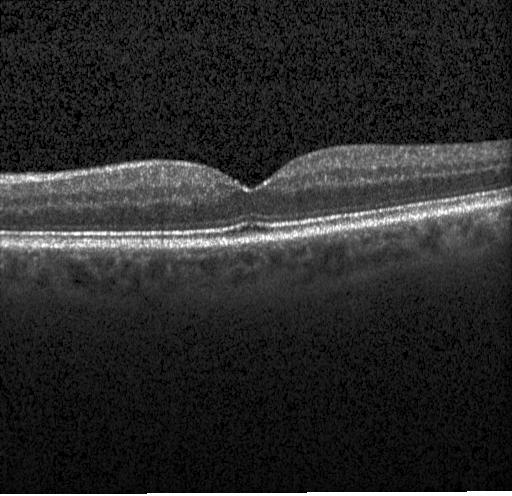
Diagnosis: neither choroidal neovascularization, diabetic macular edema, nor drusen.